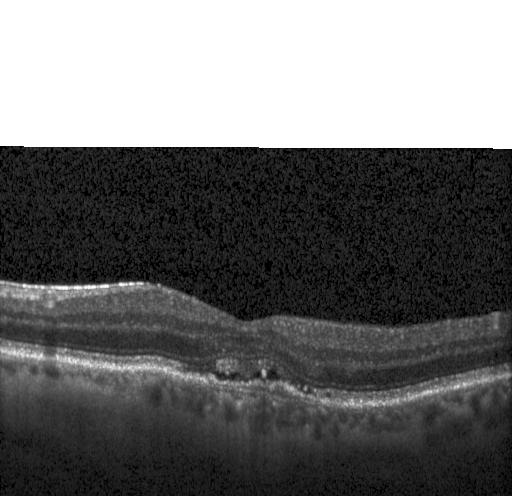

OCT line scan.
Assessment: choroidal neovascularization (CNV).